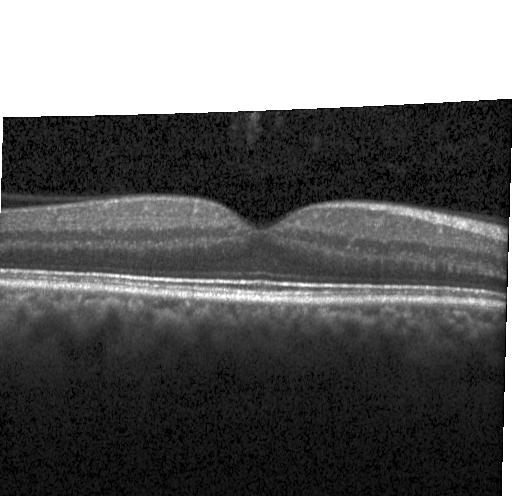 OCT scan showing no choroidal neovascularization, diabetic macular edema, or drusen.